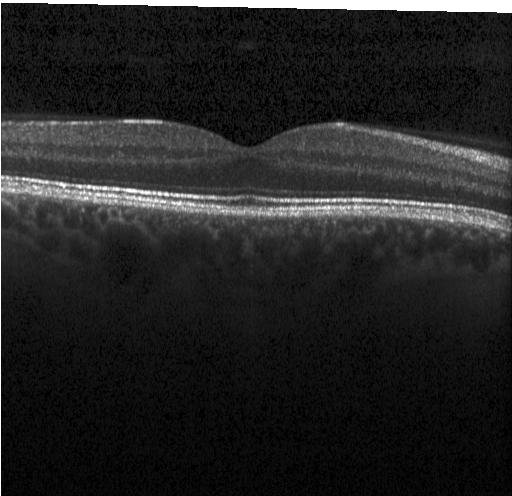 Impression: no evidence of CNV, DME, or drusen.